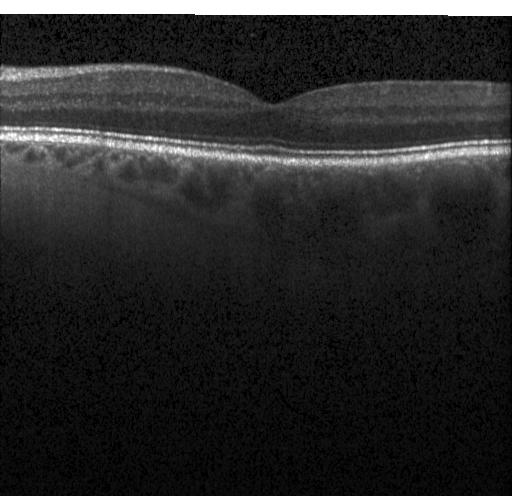 OCT B-scan, macular scan. Finding: neither choroidal neovascularization, diabetic macular edema, nor drusen.